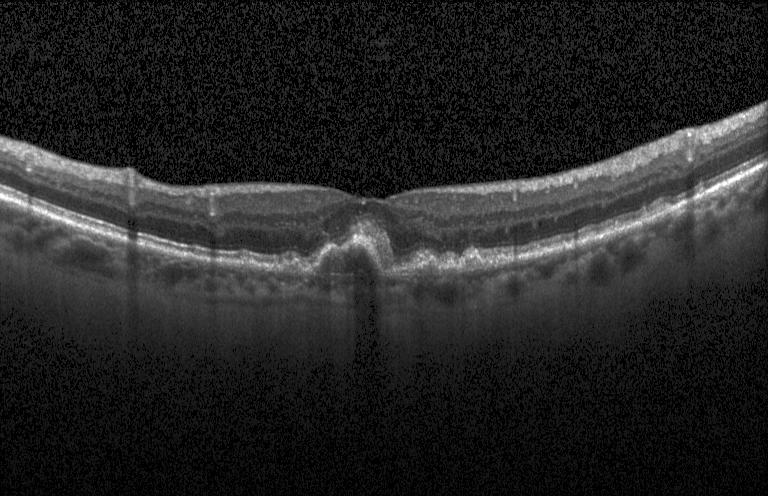 Heidelberg Spectralis, retinal OCT cross-section, SD-OCT
Choroidal neovascularization (CNV).